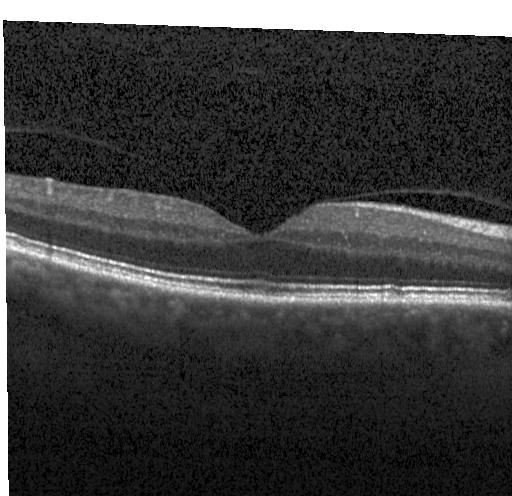

This B-scan demonstrates no choroidal neovascularization, diabetic macular edema, or drusen.